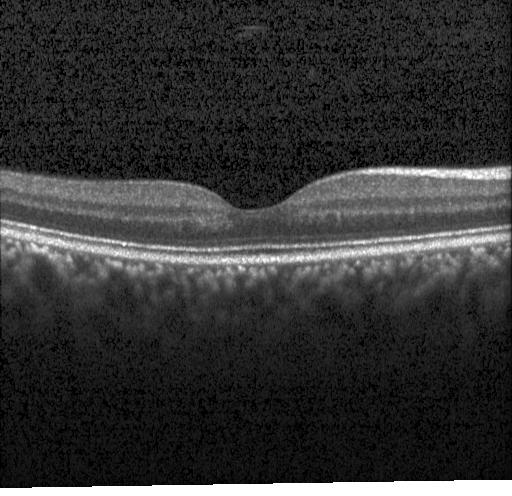
Impression: neither CNV, DME, nor drusen.